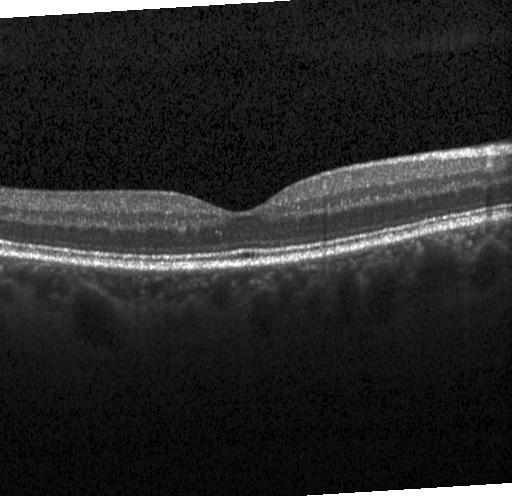

Assessment: no evidence of CNV, DME, or drusen.